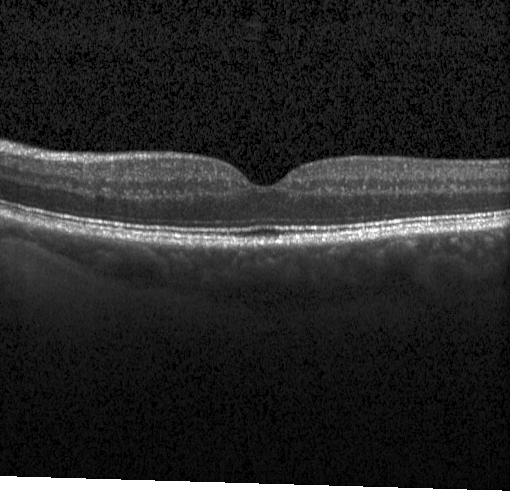
Macular OCT demonstrating no choroidal neovascularization, diabetic macular edema, or drusen.